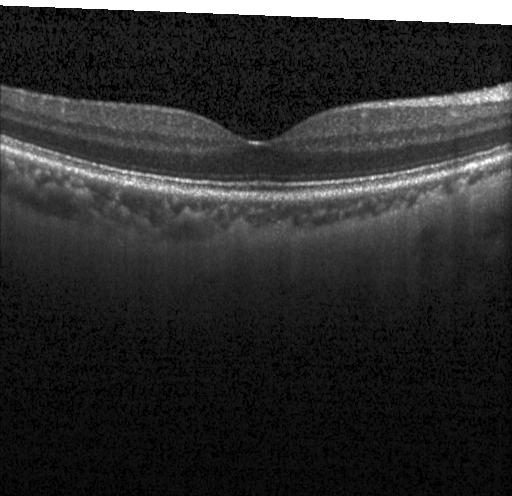

Fovea-centered. Optical coherence tomography scan
Dx: neither CNV, DME, nor drusen.